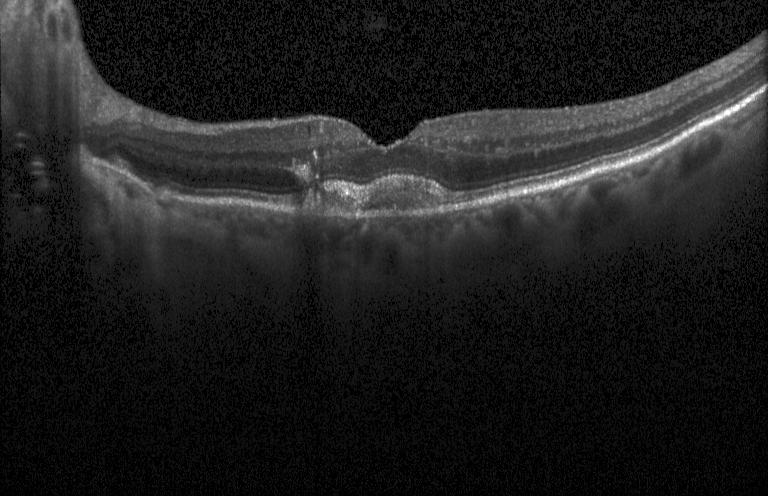
Impression: choroidal neovascularization (CNV).